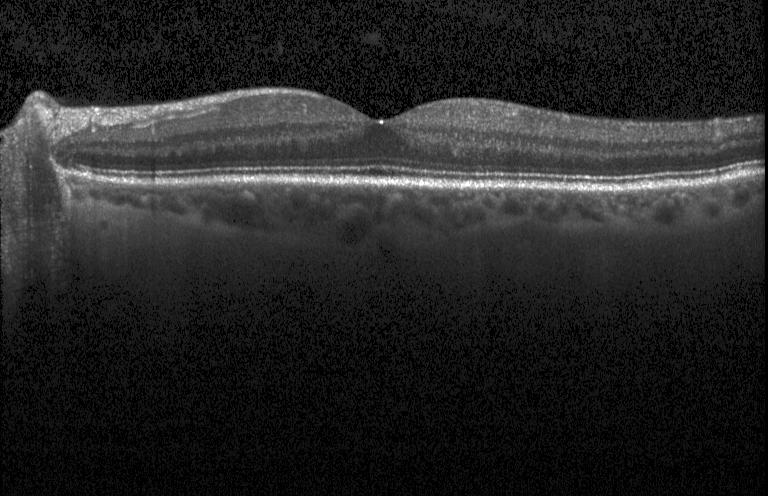

OCT line scan
Diagnosis: neither CNV, DME, nor drusen.